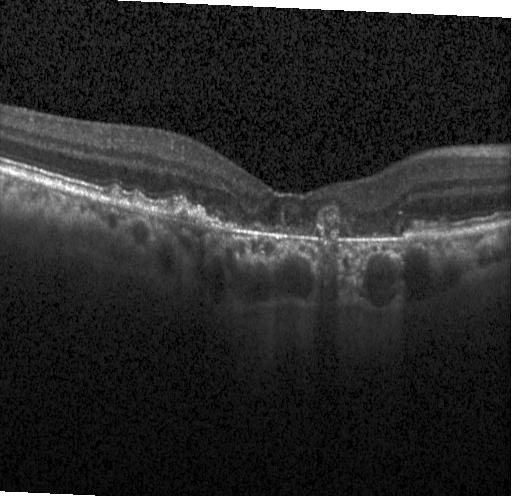

Optical coherence tomography B-scan — OCT finding: CNV.